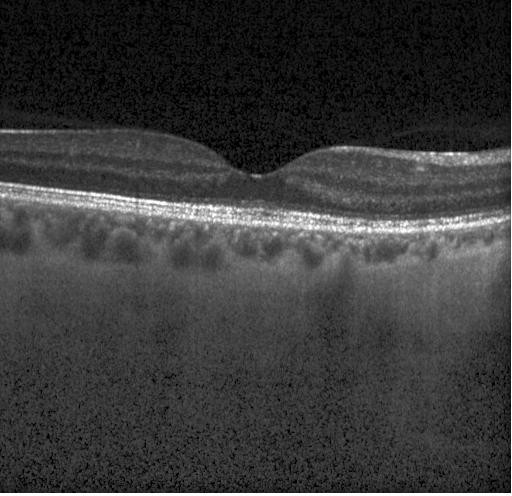
Spectral-domain OCT B-scan: no evidence of CNV, DME, or drusen.